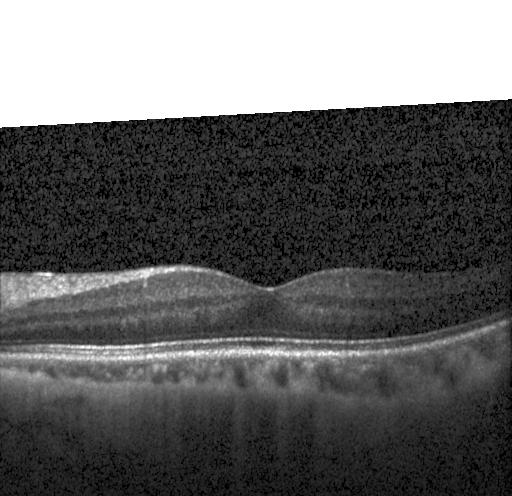

OCT line scan — The scan shows no CNV, DME, or drusen.